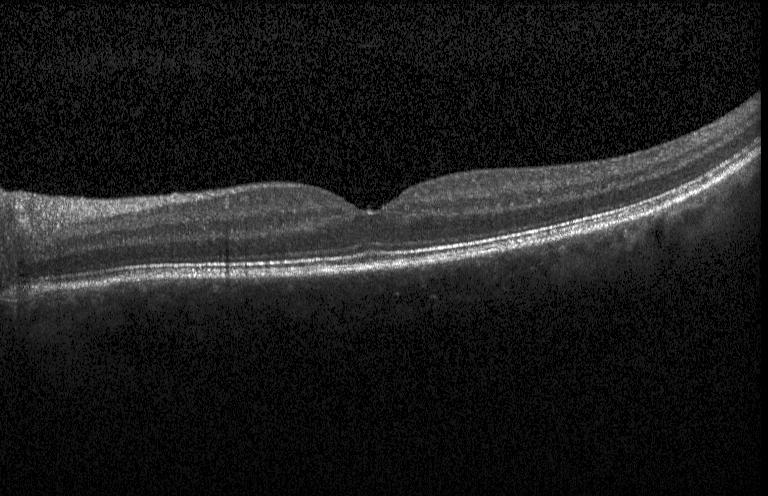
OCT B-scan; instrument: Heidelberg Spectralis
Impression: neither choroidal neovascularization, diabetic macular edema, nor drusen.